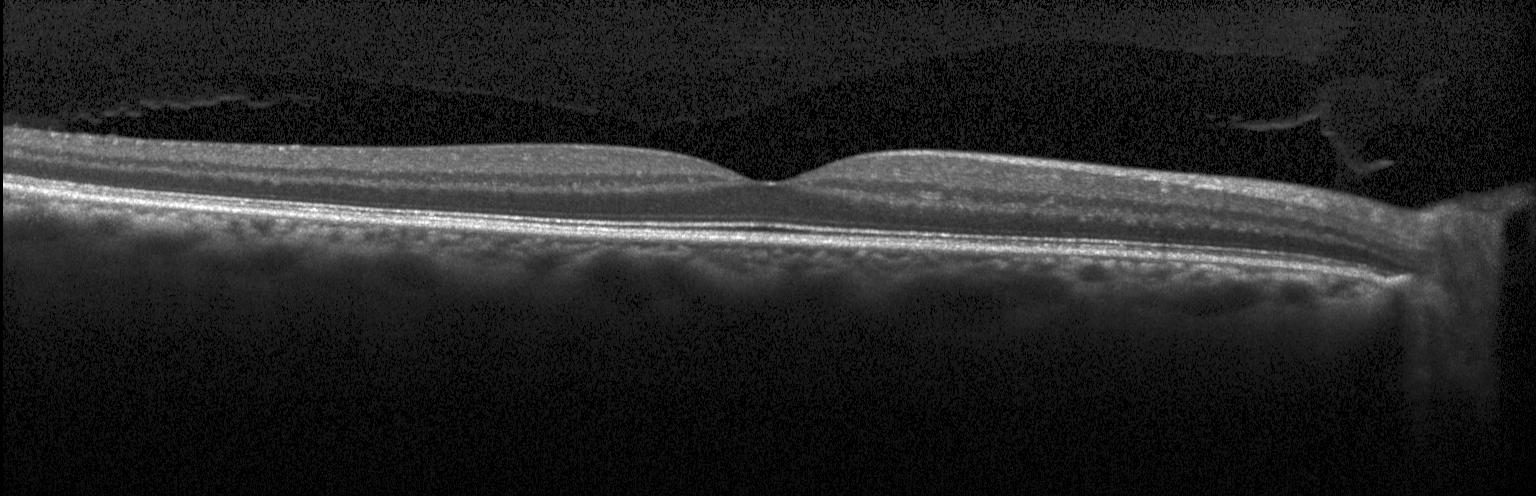

OCT B-scan
Assessment: no choroidal neovascularization, diabetic macular edema, or drusen.